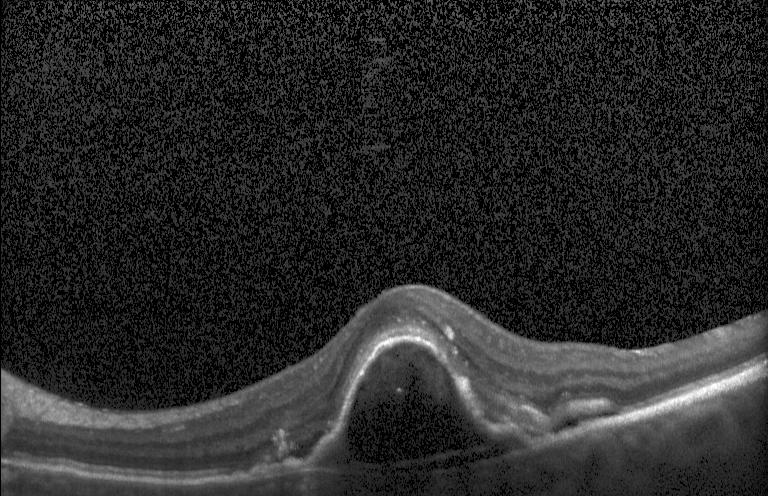
Optical coherence tomography scan. Assessment: a choroidal neovascular membrane.